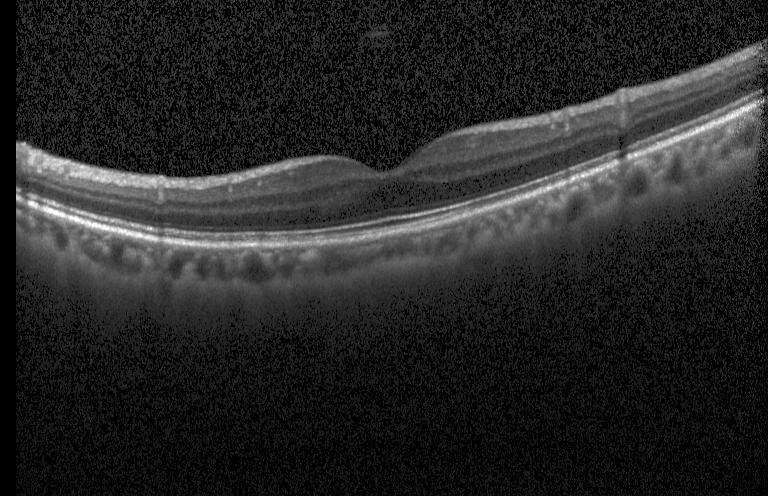
OCT B-scan showing no evidence of choroidal neovascularization, diabetic macular edema, or drusen.